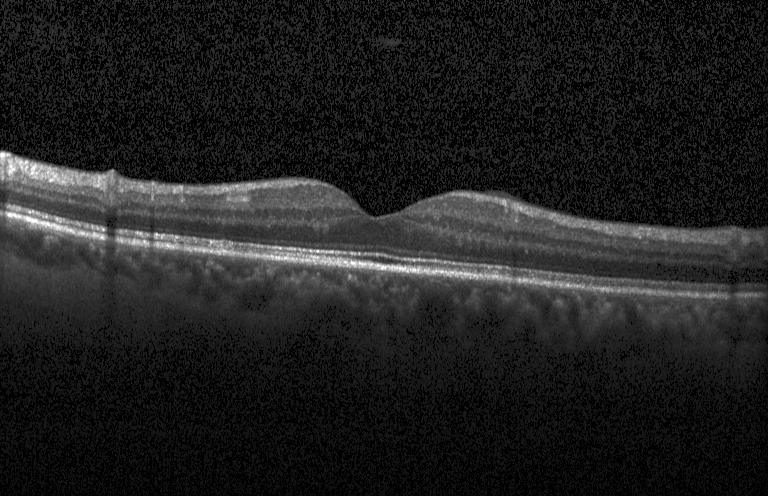

SD-OCT · macular scan · retinal OCT cross-section — Impression: no choroidal neovascularization, diabetic macular edema, or drusen.